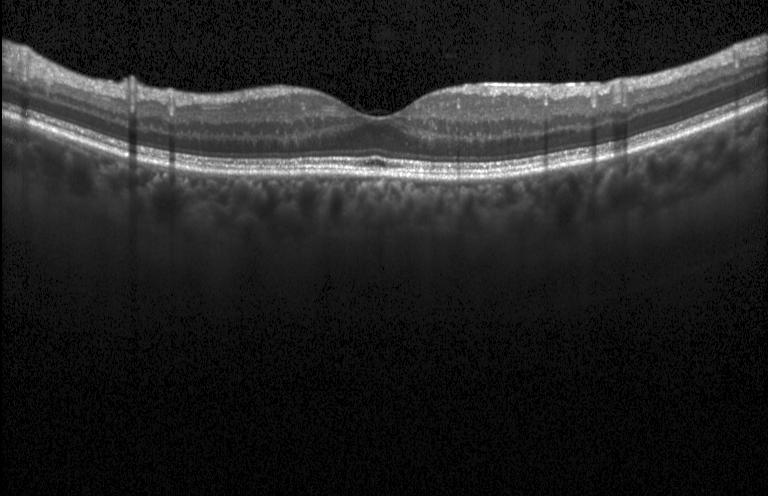 Finding: no evidence of choroidal neovascularization, diabetic macular edema, or drusen.